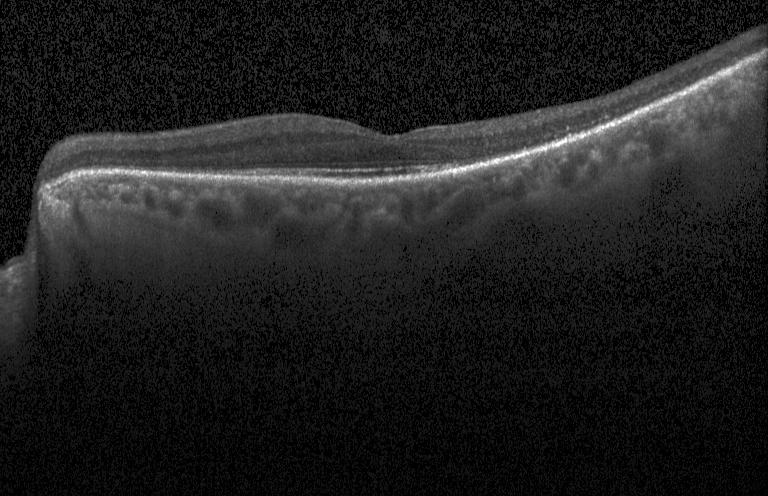

Spectral-domain OCT; through the macula; optical coherence tomography B-scan. OCT finding: no choroidal neovascularization, no diabetic macular edema, and no drusen.